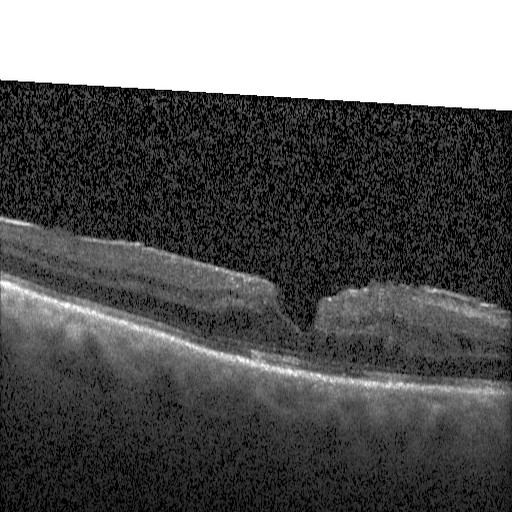 Instrument: Heidelberg Spectralis · fovea-centered · retinal OCT cross-section — Finding: diabetic macular edema (DME).